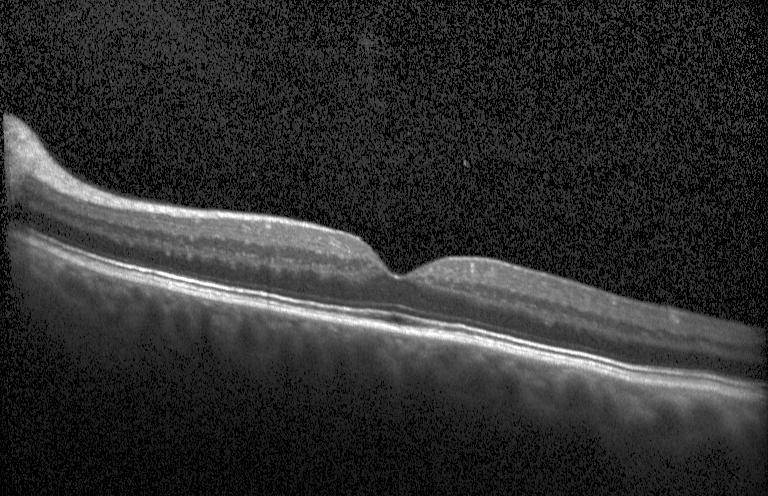

Retinal OCT cross-section showing neither CNV, DME, nor drusen.